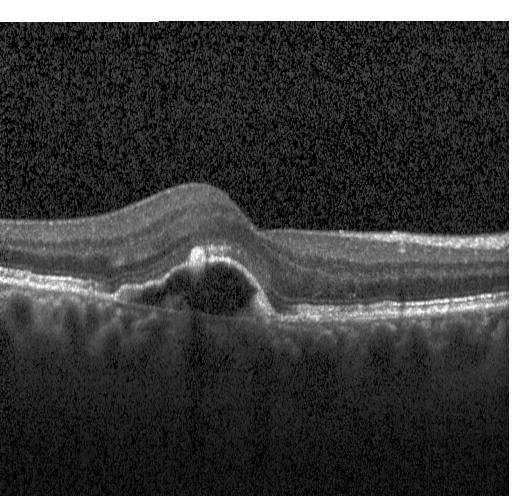

Through the macula; spectral-domain optical coherence tomography; retinal OCT B-scan — Dx: choroidal neovascularization.